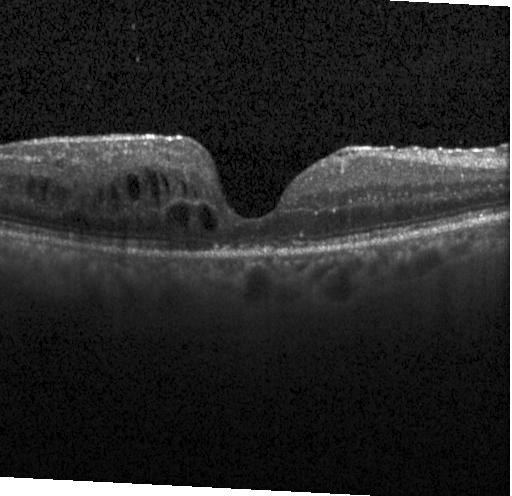

This B-scan demonstrates diabetic macular edema (DME).